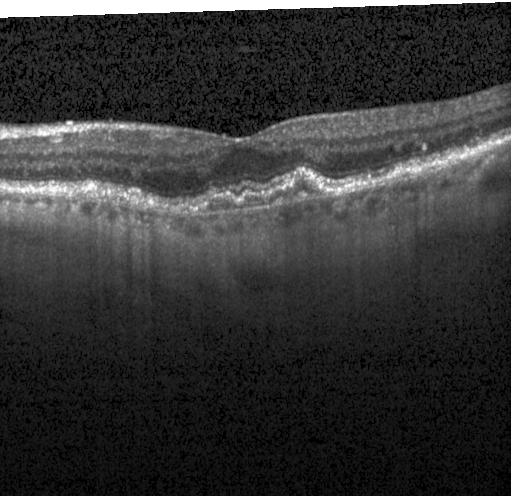

Acquired on a Heidelberg Spectralis. Spectral-domain optical coherence tomography. Optical coherence tomography scan. Centered on the fovea.
Macular OCT: a choroidal neovascular membrane.